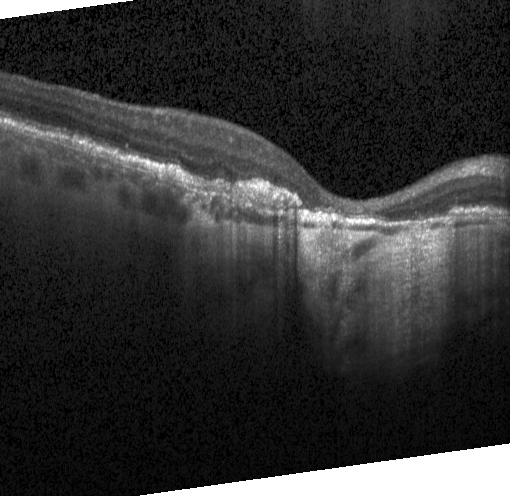
Heidelberg Spectralis · optical coherence tomography B-scan · spectral-domain optical coherence tomography.
A choroidal neovascular membrane.